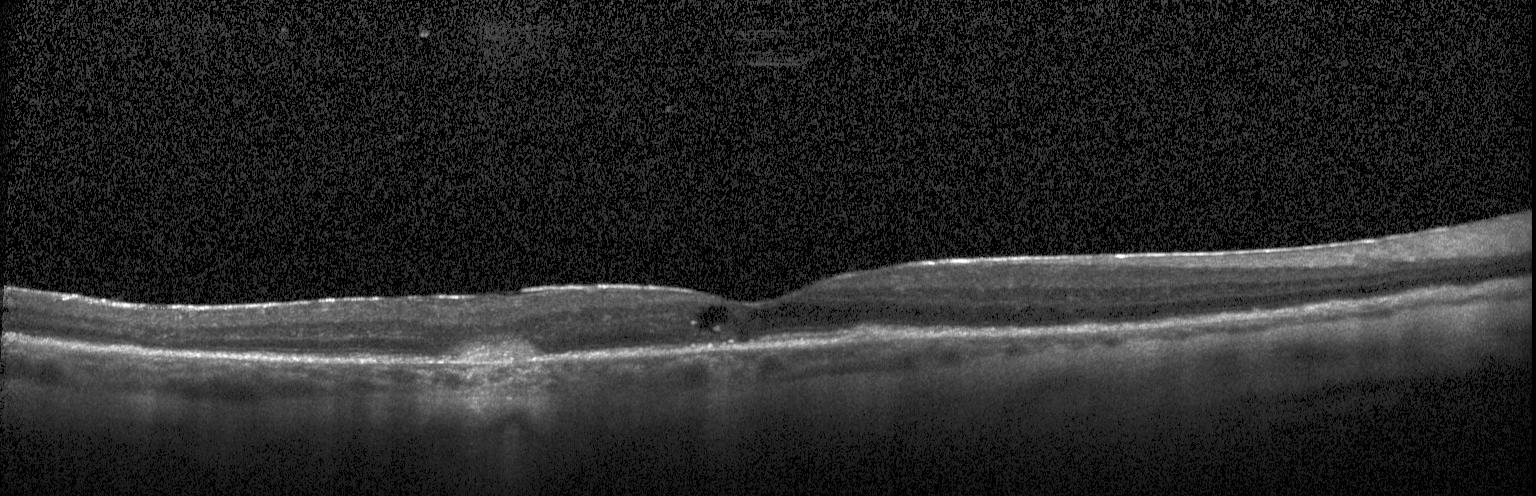
Dx: choroidal neovascularization (CNV).